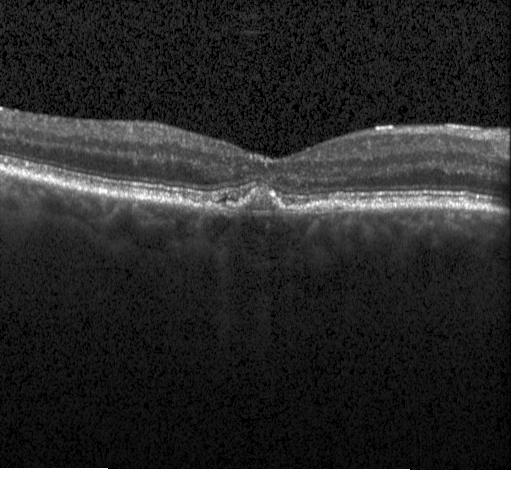 OCT finding: CNV.